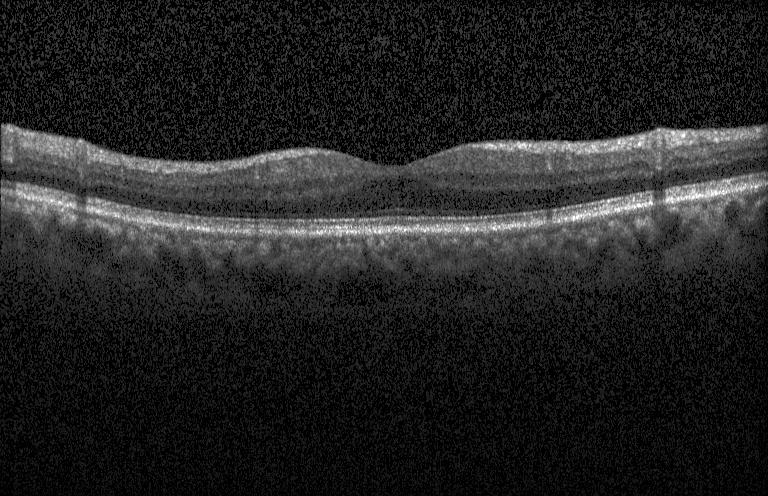 Retinal OCT cross-section.
Diagnosis: no choroidal neovascularization, no diabetic macular edema, and no drusen.